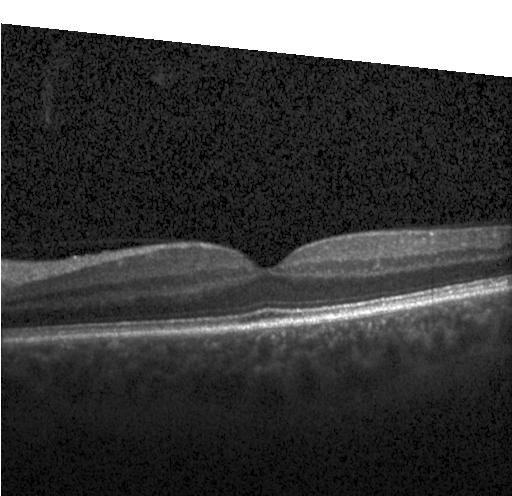 Assessment: no choroidal neovascularization, diabetic macular edema, or drusen.